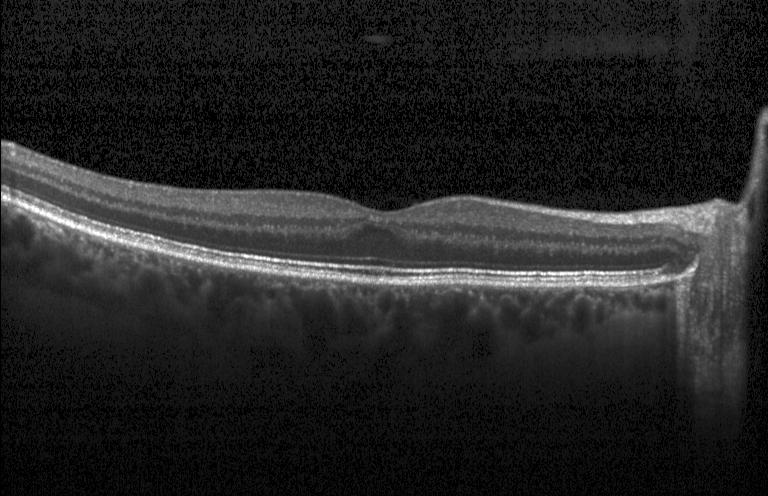 This B-scan demonstrates no evidence of choroidal neovascularization, diabetic macular edema, or drusen.